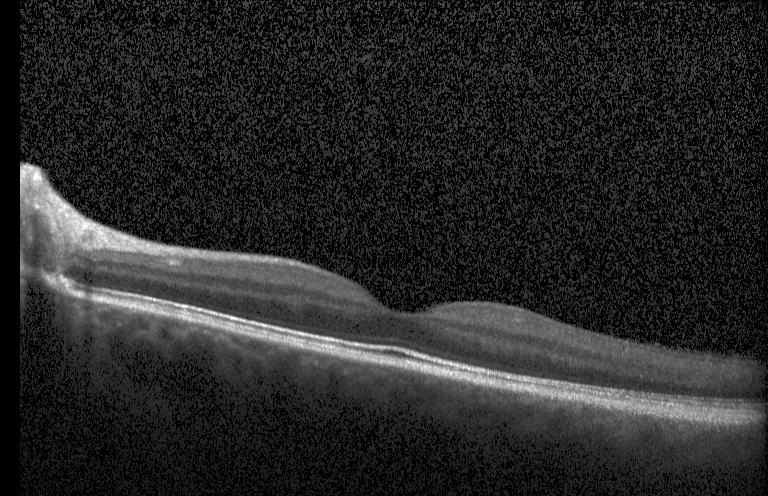

Acquired on a Heidelberg Spectralis · spectral-domain optical coherence tomography · retinal OCT B-scan · through the macula. Finding: no choroidal neovascularization, diabetic macular edema, or drusen.